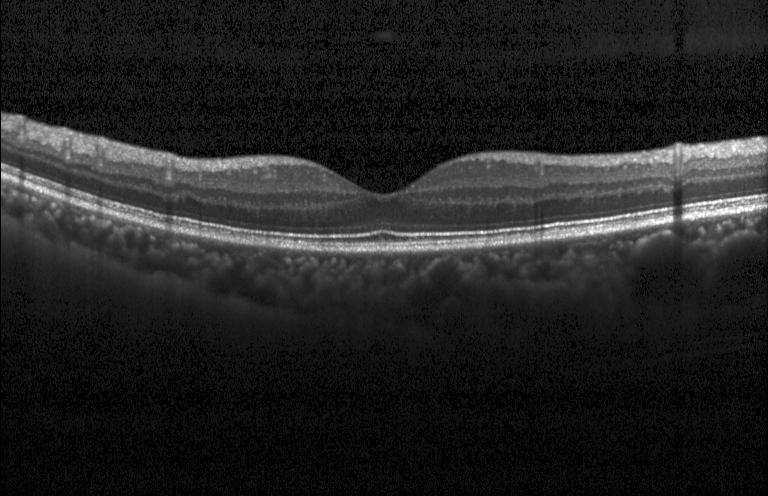

Assessment: no CNV, no DME, and no drusen.